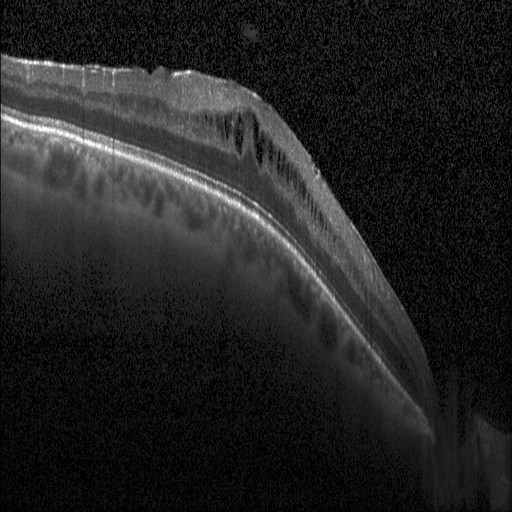 Assessment: diabetic macular edema.